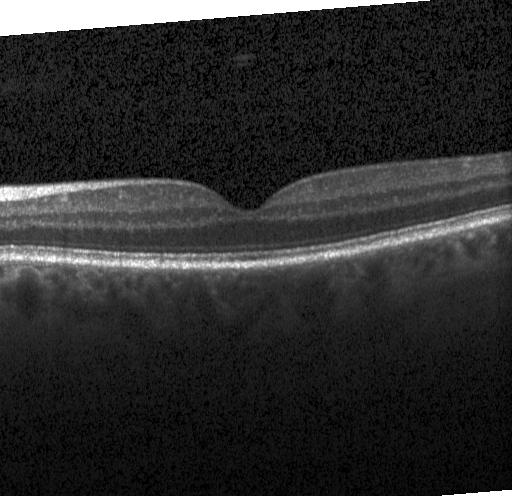 The scan shows no evidence of CNV, DME, or drusen.